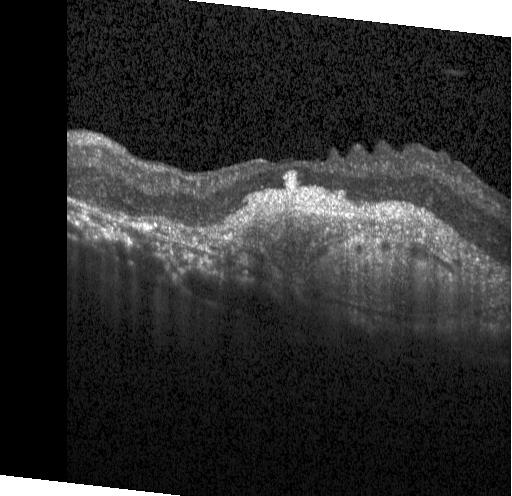
Spectral-domain optical coherence tomography · OCT line scan. Finding: CNV.